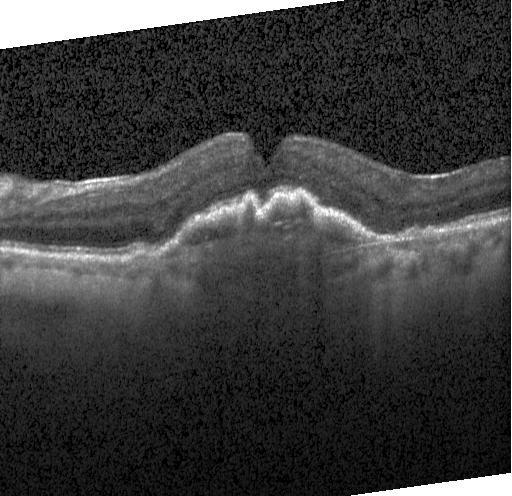

Retinal OCT cross-section · SD-OCT
Assessment: a choroidal neovascular membrane.